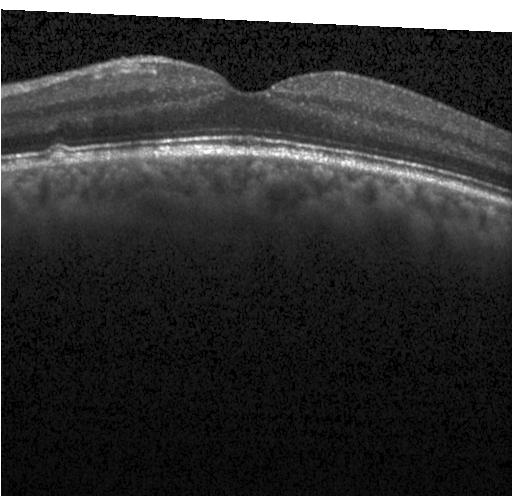 Finding: no choroidal neovascularization, no diabetic macular edema, and no drusen.